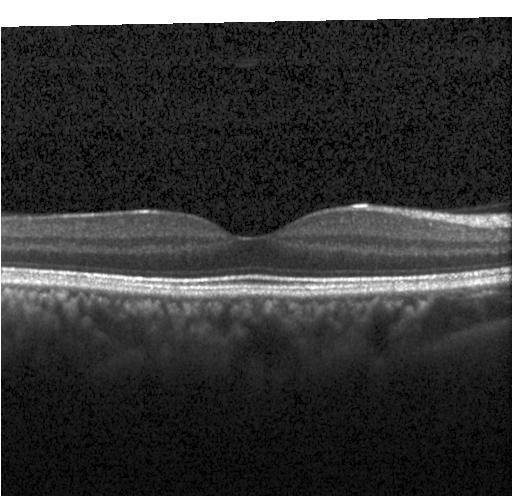
The scan shows no choroidal neovascularization, no diabetic macular edema, and no drusen.